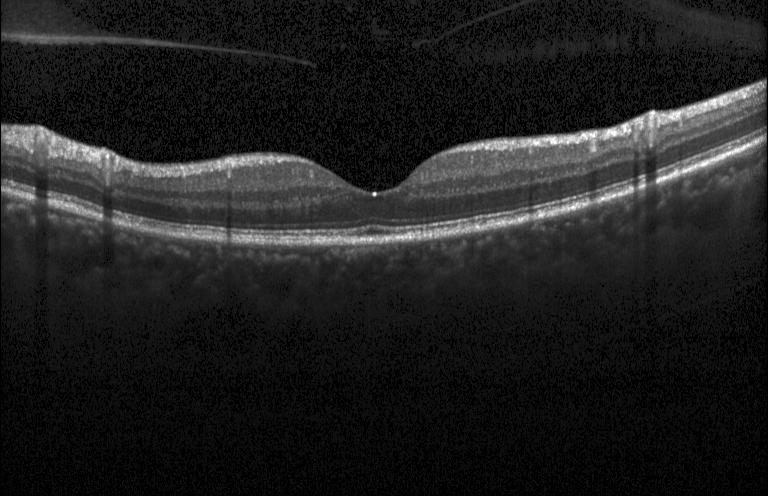
Spectral-domain OCT. Instrument: Heidelberg Spectralis. Retinal OCT cross-section.
This B-scan demonstrates no choroidal neovascularization, diabetic macular edema, or drusen.